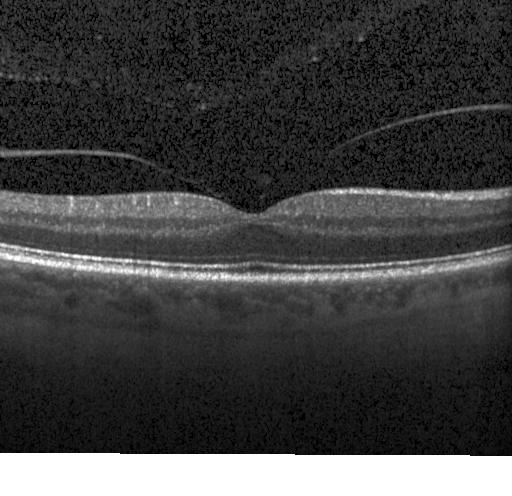

Heidelberg Spectralis OCT system · horizontal scan through the fovea · retinal OCT cross-section · spectral-domain OCT. Impression: no evidence of choroidal neovascularization, diabetic macular edema, or drusen.